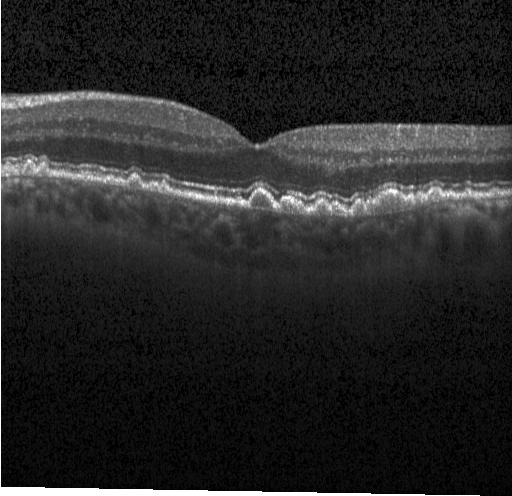

Heidelberg Spectralis · retinal OCT cross-section · through the macula · spectral-domain OCT — Impression: drusen.